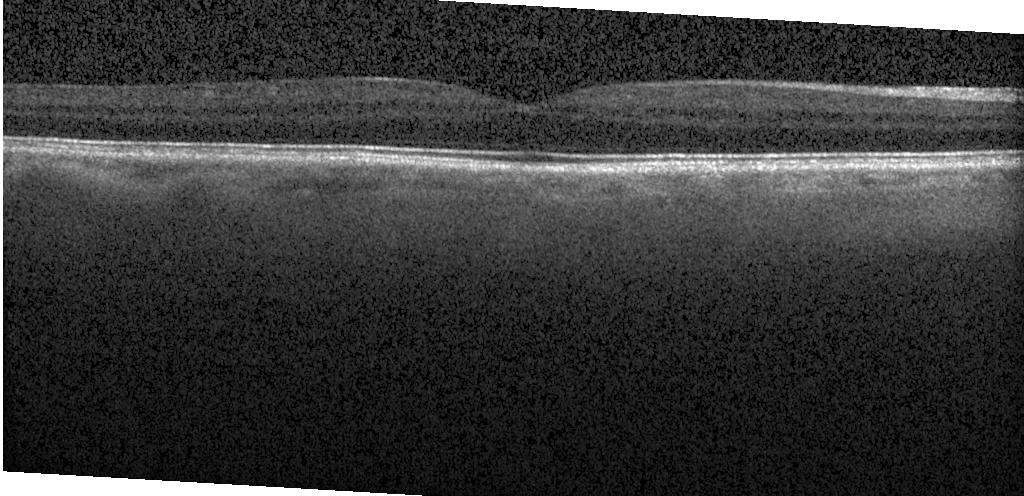

OCT line scan · SD-OCT · acquired on a Heidelberg Spectralis · macular scan. Macular OCT: no choroidal neovascularization, no diabetic macular edema, and no drusen.